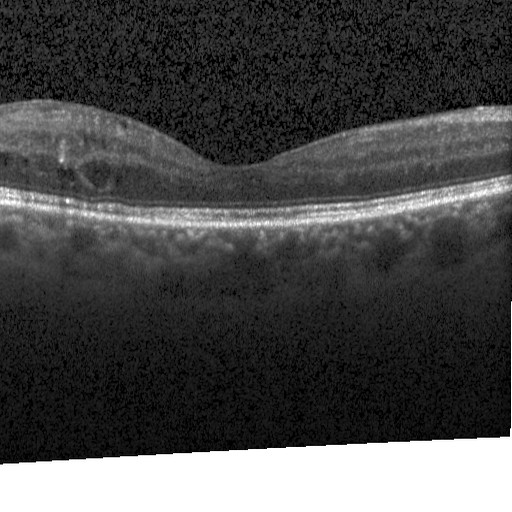

Macular OCT demonstrating DME.